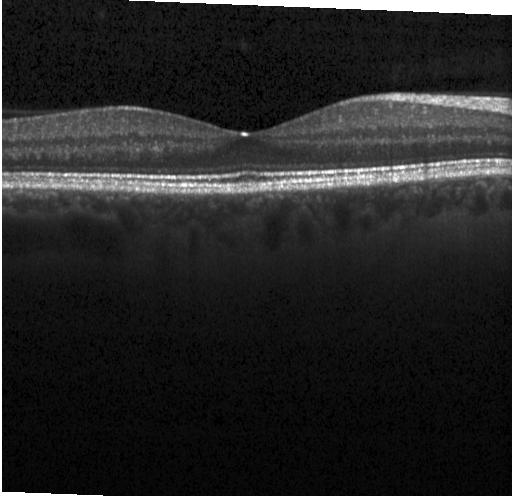 SD-OCT. Retinal OCT cross-section. Dx: no evidence of CNV, DME, or drusen.